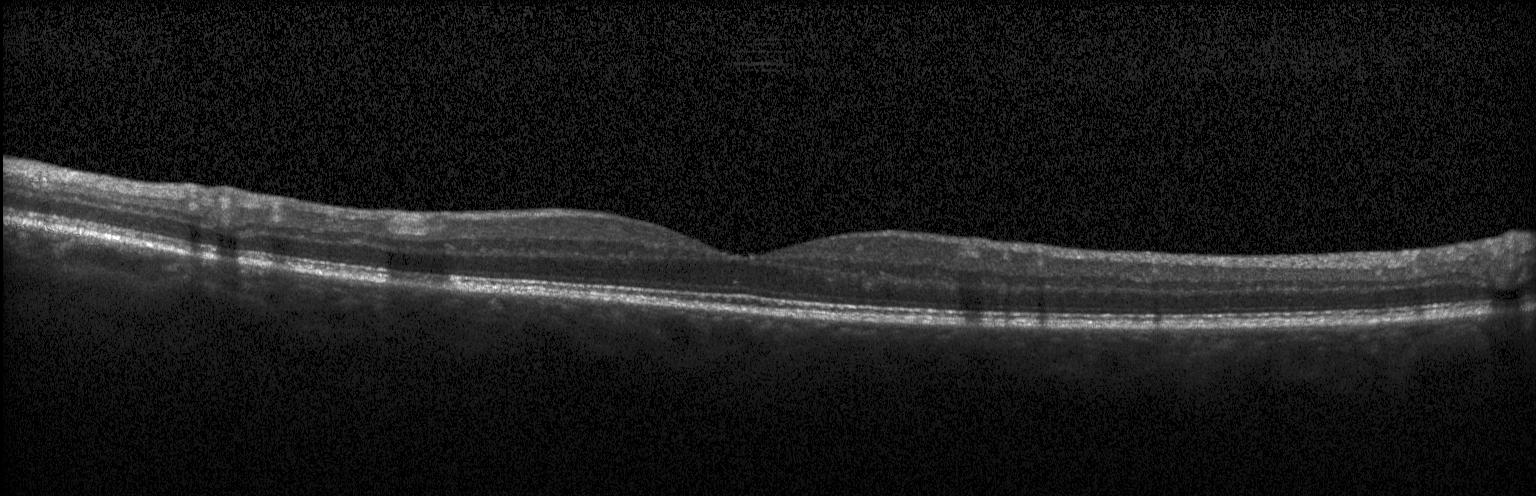
Instrument: Heidelberg Spectralis · OCT line scan
No choroidal neovascularization, no diabetic macular edema, and no drusen.